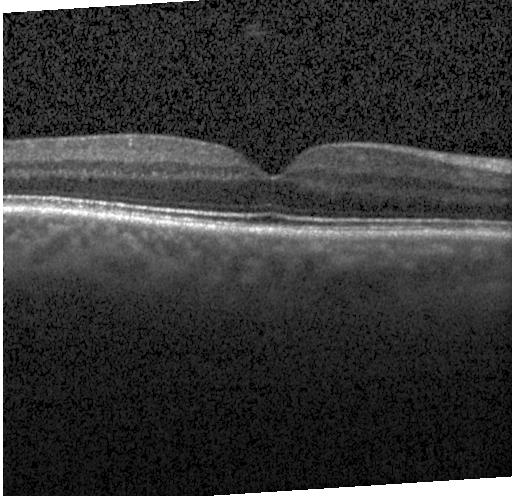 Dx: no choroidal neovascularization, diabetic macular edema, or drusen.